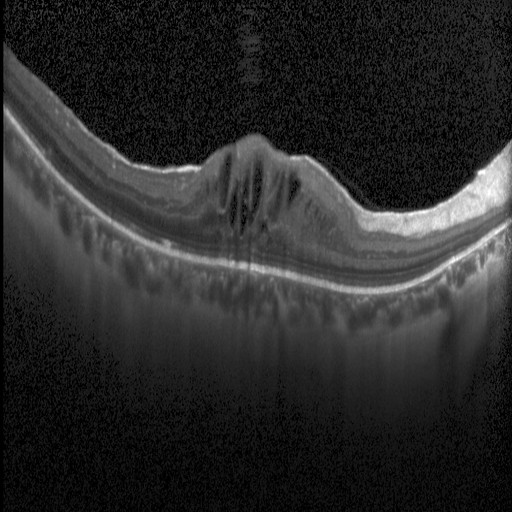 Spectral-domain OCT B-scan: diabetic macular edema.